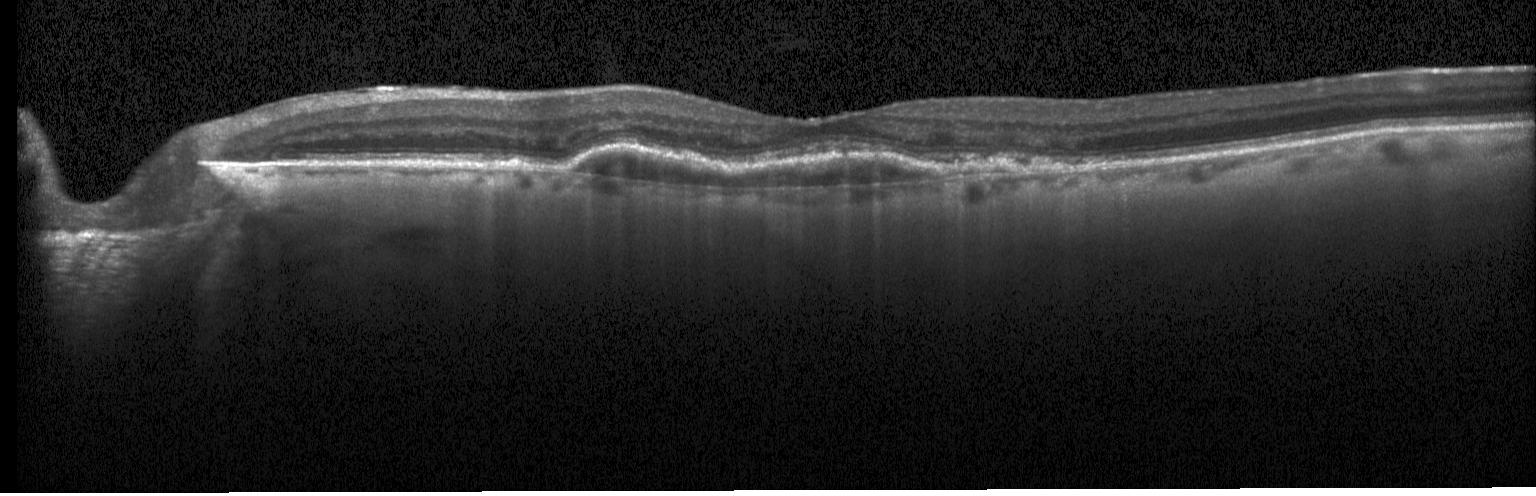 Optical coherence tomography B-scan. Acquired on a Heidelberg Spectralis. Fovea-centered. Finding: CNV.